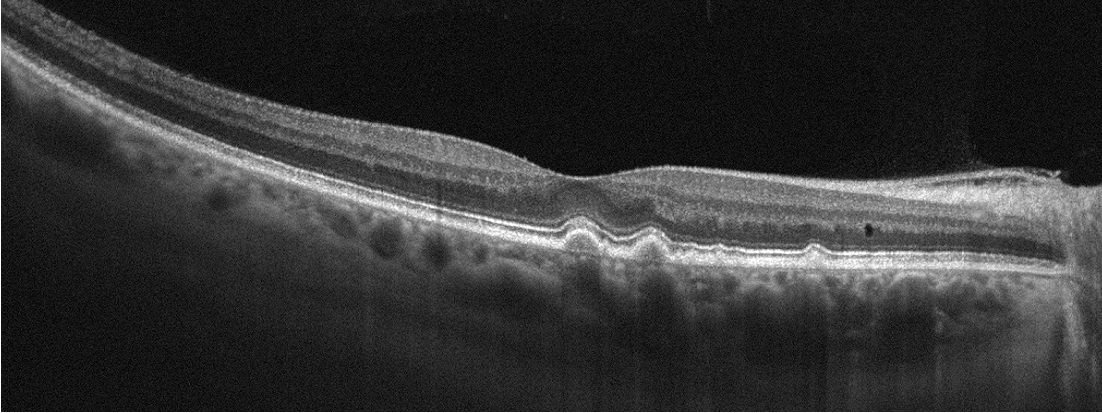
Optical coherence tomography scan. Assessment: age-related macular degeneration.